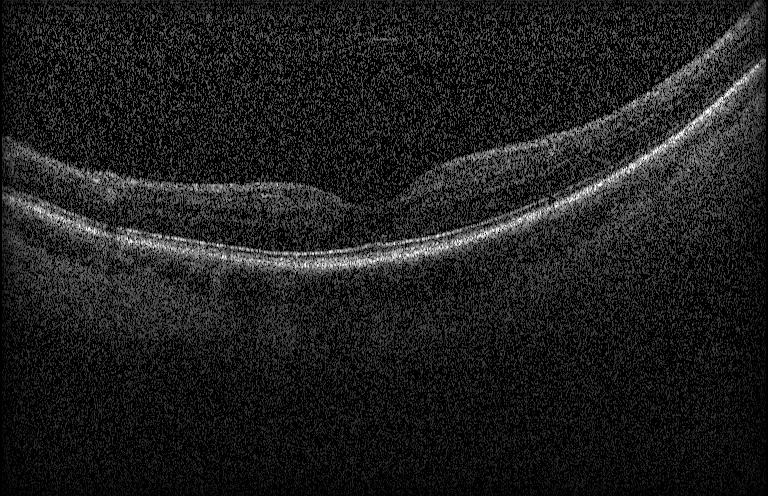
Through the macula · Heidelberg Spectralis OCT system · OCT line scan
The scan shows no choroidal neovascularization, diabetic macular edema, or drusen.